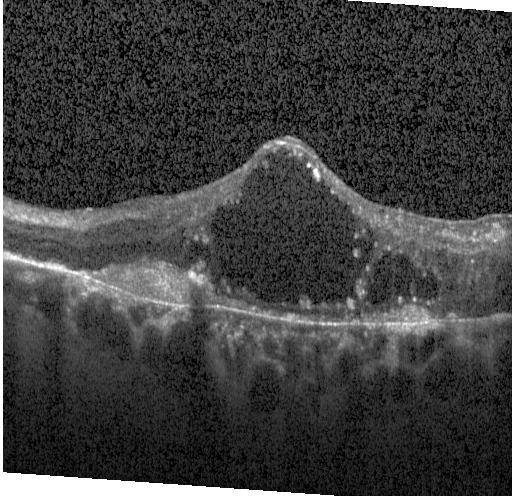 Spectral-domain optical coherence tomography; Heidelberg Spectralis; retinal OCT cross-section — Diagnosis: a choroidal neovascular membrane.